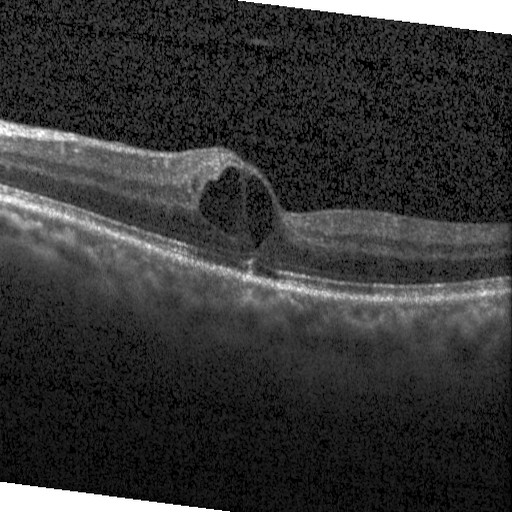
The scan shows diabetic macular edema.